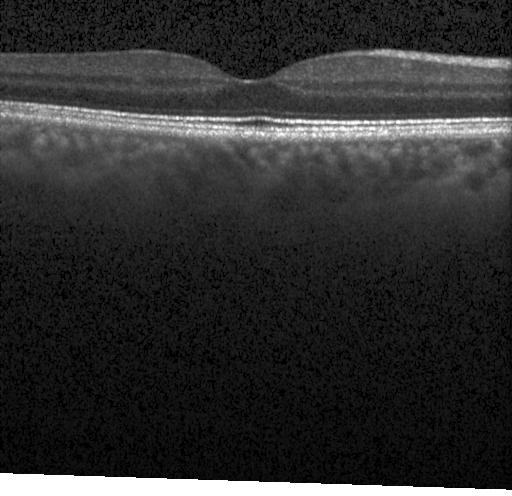 OCT B-scan, spectral-domain optical coherence tomography. The scan shows no choroidal neovascularization, no diabetic macular edema, and no drusen.